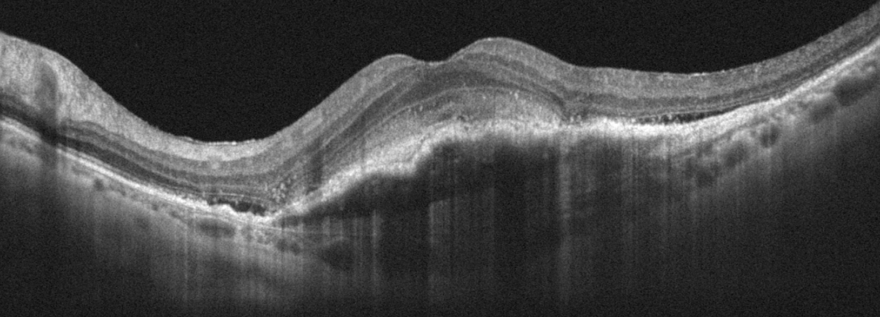

OCT B-scan showing age-related macular degeneration (AMD).